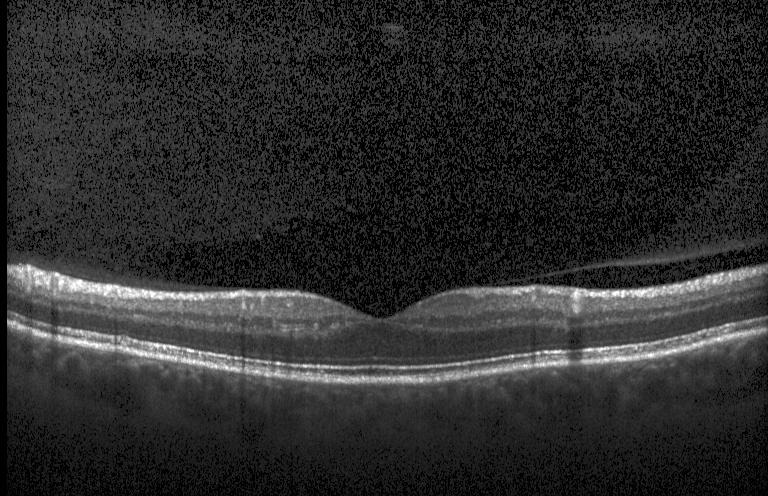
OCT B-scan.
Impression: no evidence of choroidal neovascularization, diabetic macular edema, or drusen.